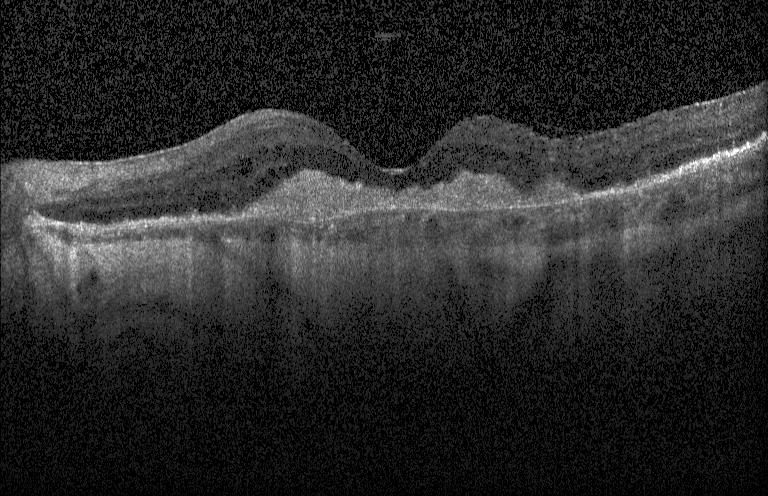

SD-OCT, retinal OCT B-scan, through the macula
Finding: choroidal neovascularization (CNV).